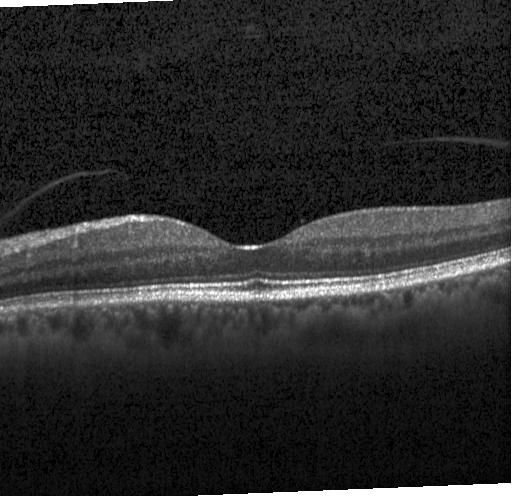

The scan shows no evidence of choroidal neovascularization, diabetic macular edema, or drusen.